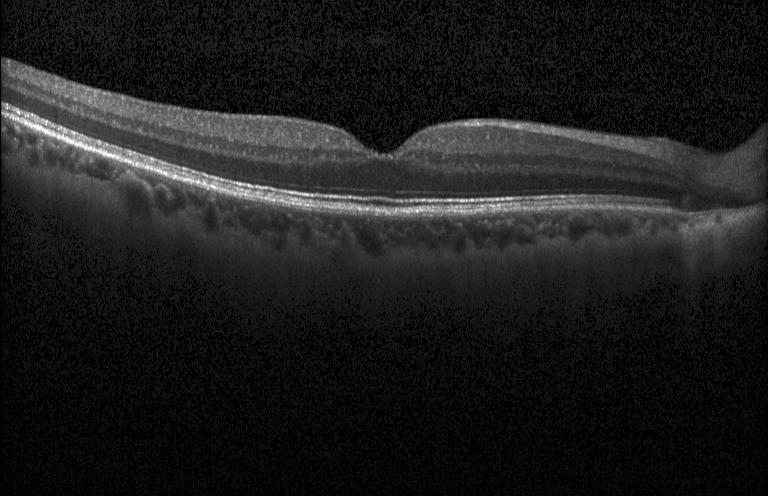

Instrument: Heidelberg Spectralis · macular scan · retinal OCT cross-section · spectral-domain OCT — OCT finding: no CNV, no DME, and no drusen.